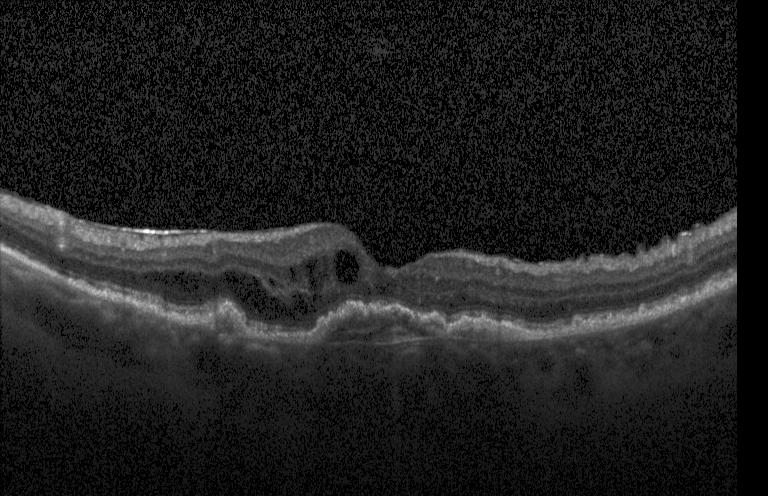
Optical coherence tomography scan. Centered on the fovea. Heidelberg Spectralis. Diagnosis: choroidal neovascularization (CNV).